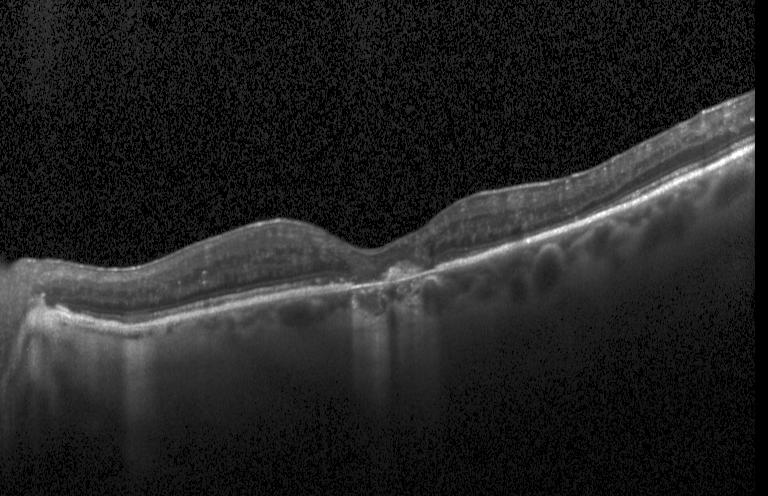

Impression: a choroidal neovascular membrane.